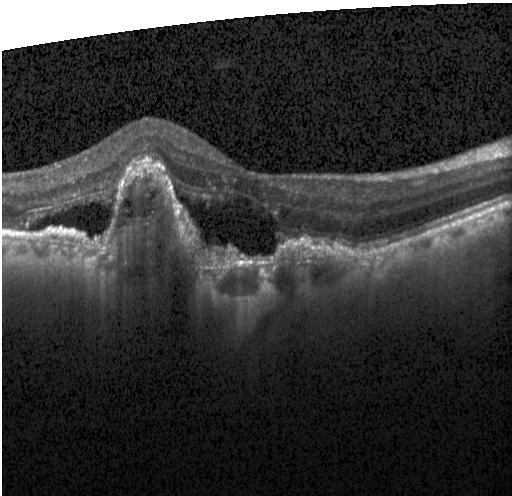
Dx: a choroidal neovascular membrane.